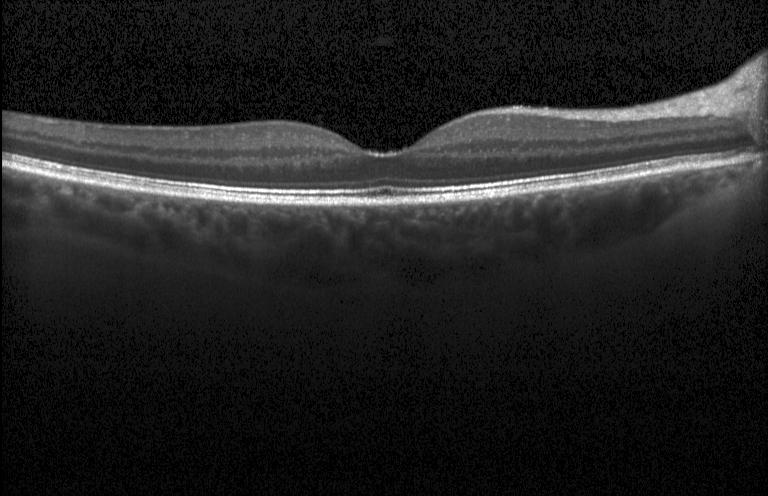
OCT finding: neither choroidal neovascularization, diabetic macular edema, nor drusen.